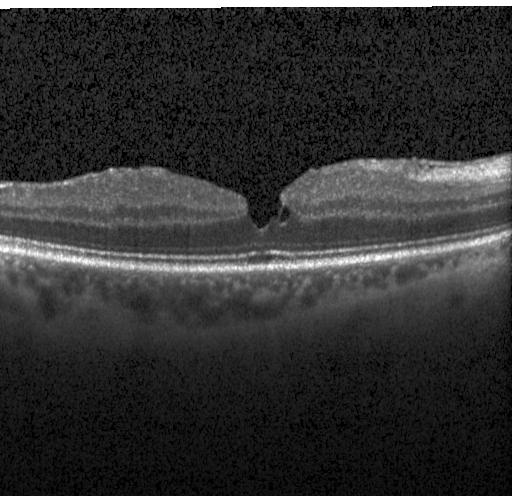
Instrument: Heidelberg Spectralis · through the macula · OCT line scan · spectral-domain OCT.
Assessment: diabetic macular edema (DME).